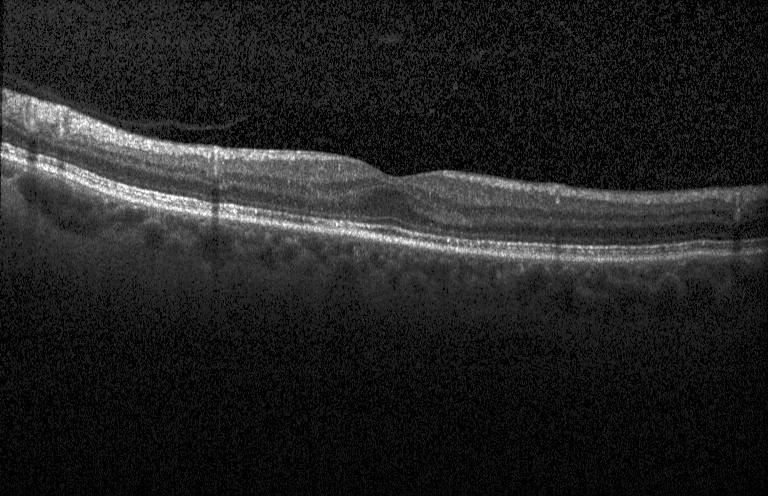

OCT B-scan showing no choroidal neovascularization, diabetic macular edema, or drusen.